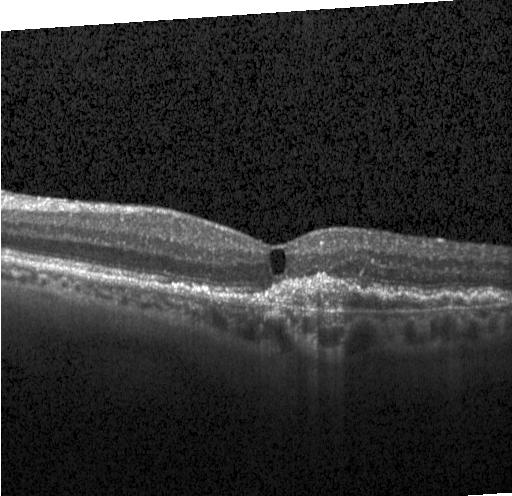 Spectral-domain OCT; retinal OCT B-scan — Assessment: a choroidal neovascular membrane.